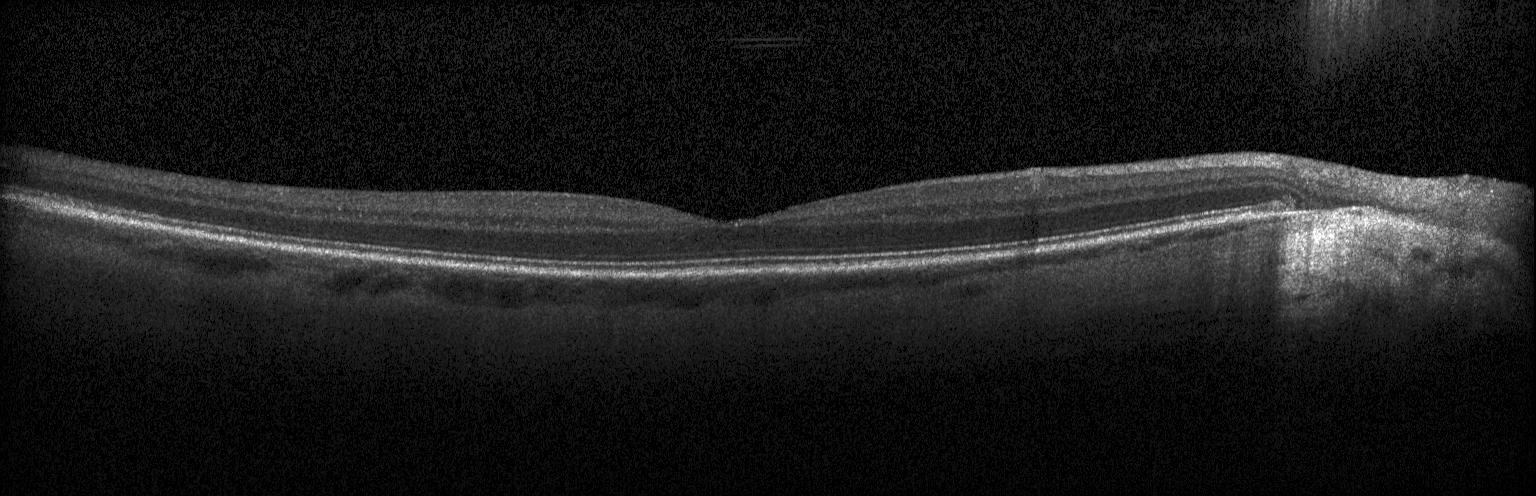
Centered on the fovea · retinal OCT B-scan — Finding: no CNV, no DME, and no drusen.